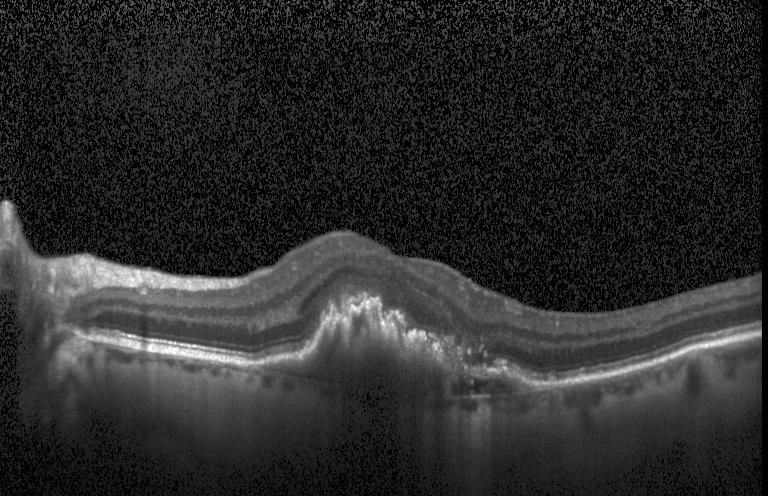

Heidelberg Spectralis, optical coherence tomography scan, spectral-domain optical coherence tomography. Finding: a choroidal neovascular membrane.